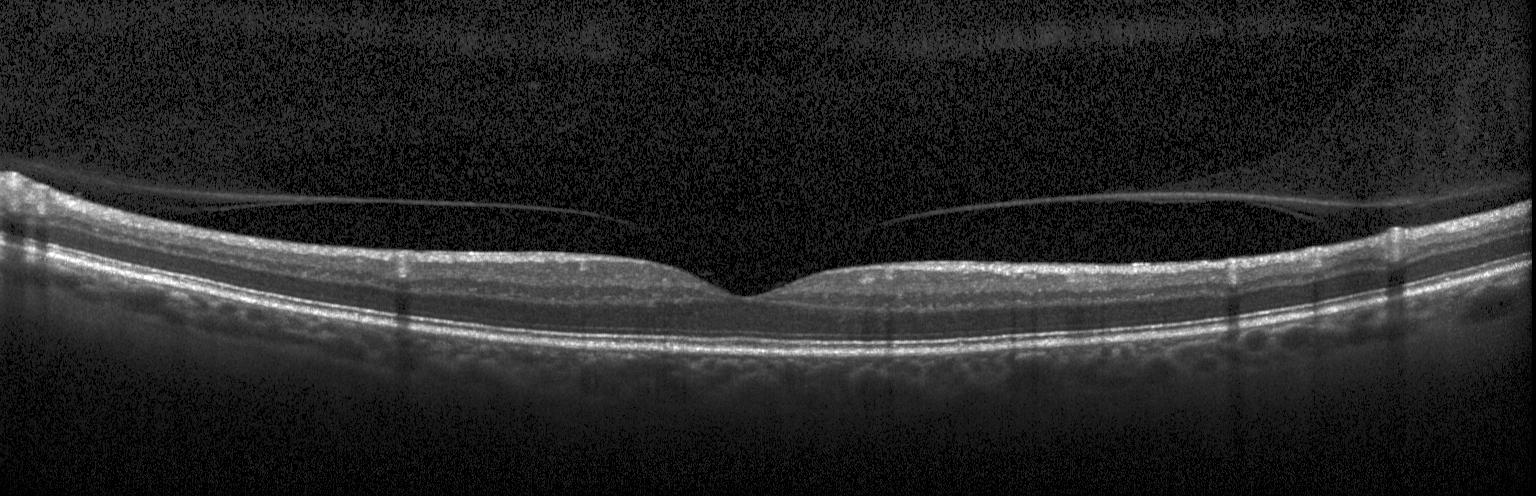
Diagnosis: no CNV, DME, or drusen.